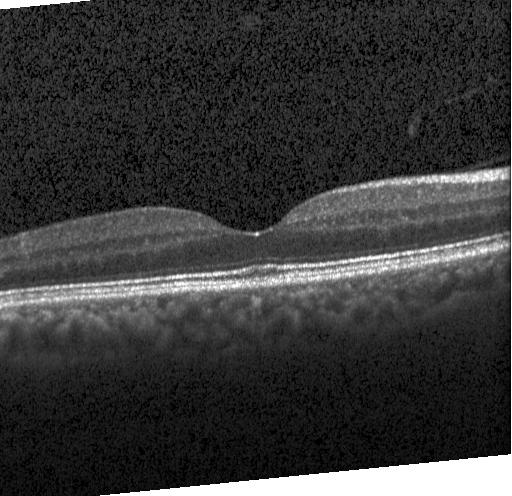

Spectral-domain OCT, retinal OCT cross-section — OCT finding: no evidence of choroidal neovascularization, diabetic macular edema, or drusen.